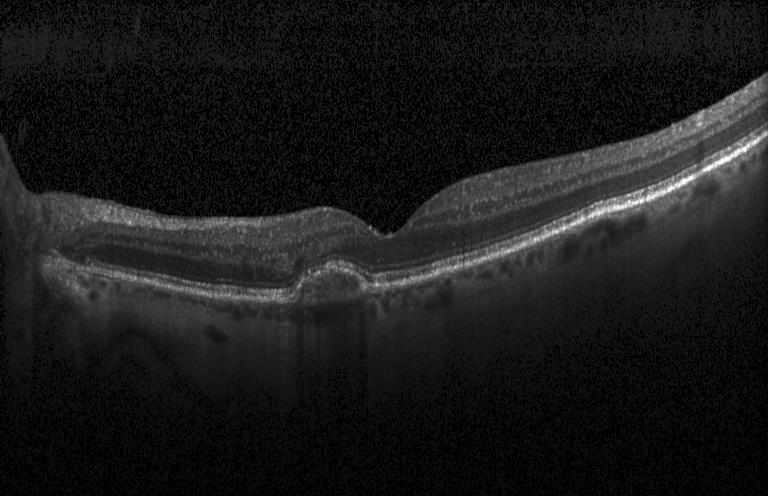
Retinal OCT B-scan. Diagnosis: a choroidal neovascular membrane.